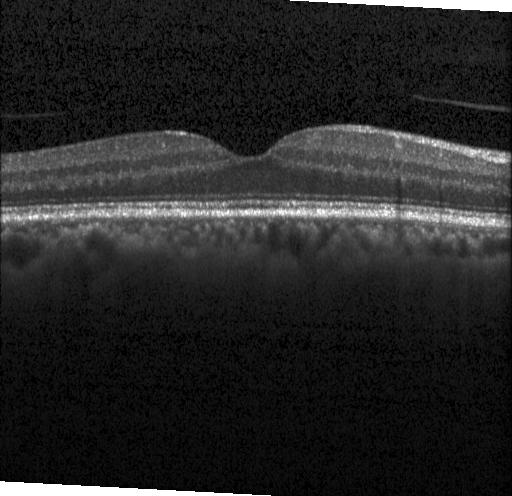

OCT B-scan showing neither choroidal neovascularization, diabetic macular edema, nor drusen.